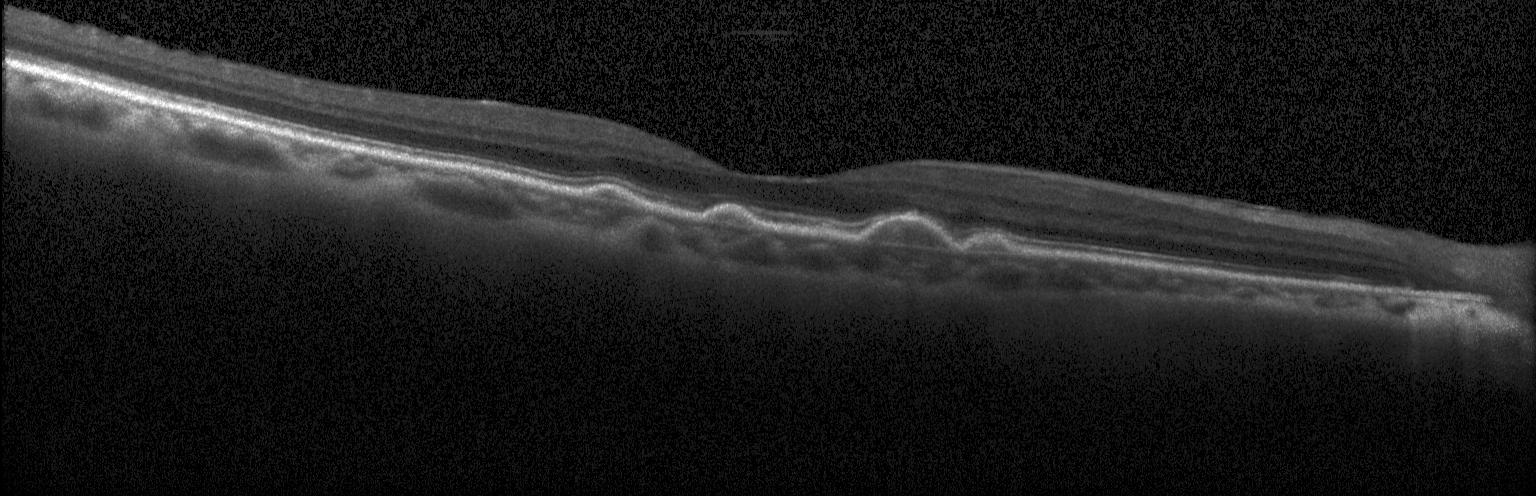
Macular OCT demonstrating drusen.